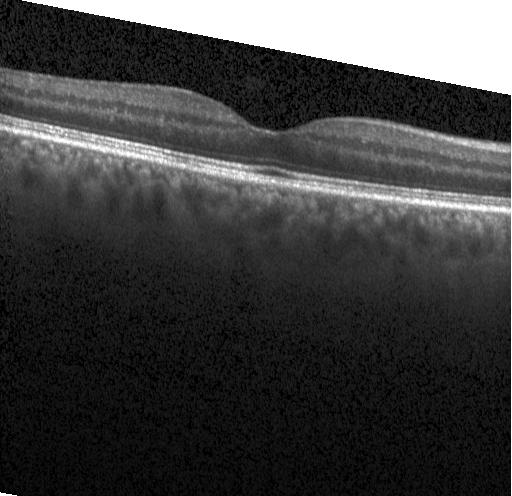
Finding: no CNV, DME, or drusen.